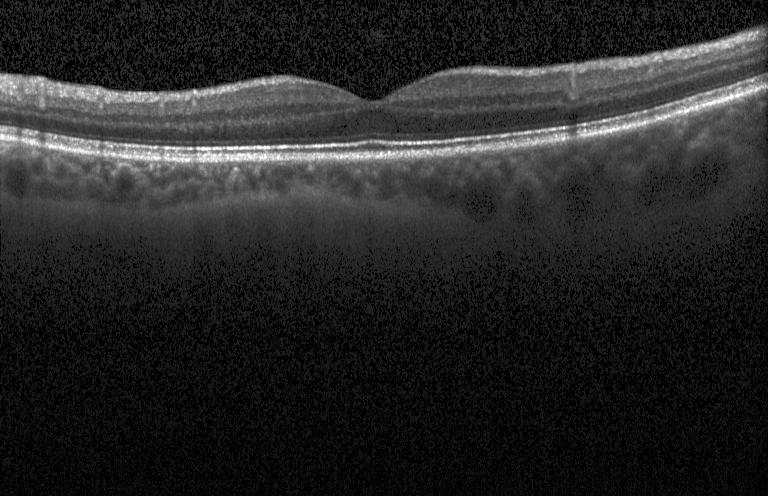
OCT scan showing no CNV, DME, or drusen.